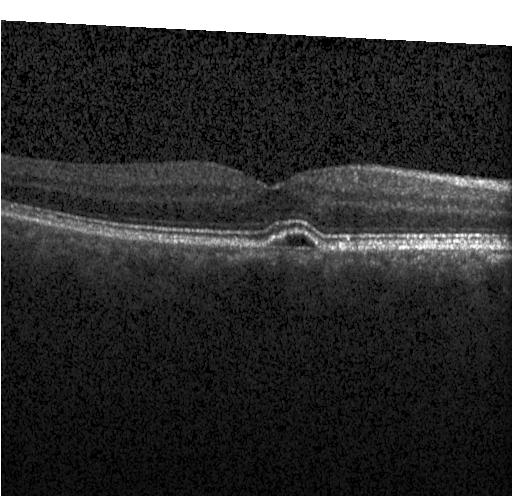 Retinal OCT B-scan.
Impression: choroidal neovascularization (CNV).